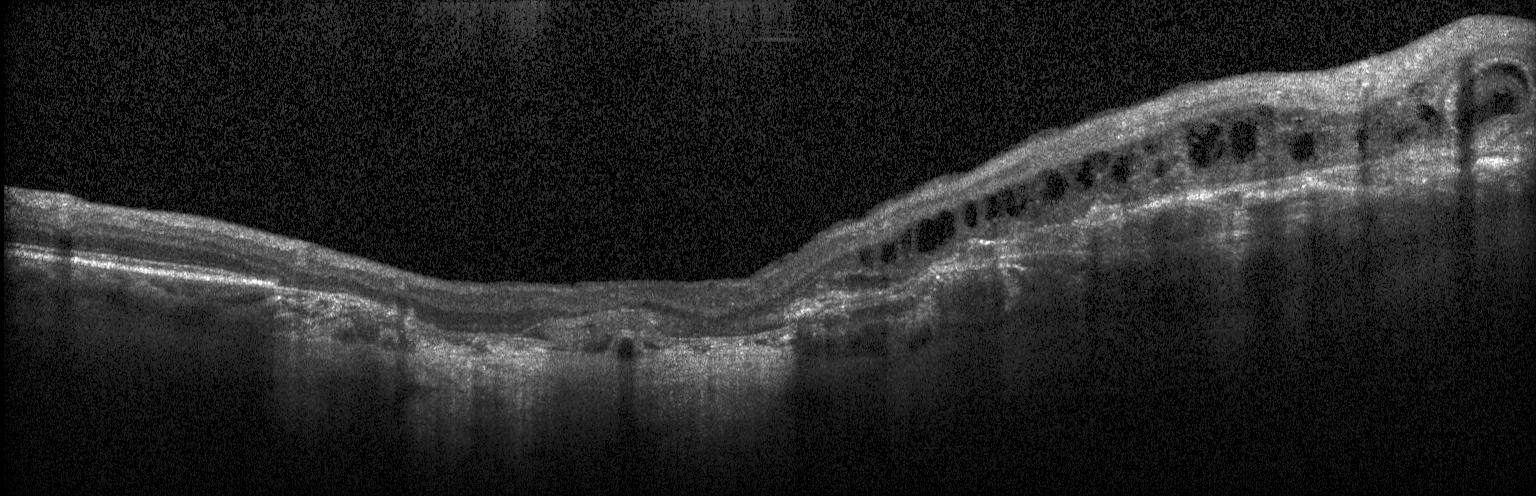

Retinal OCT B-scan. Instrument: Heidelberg Spectralis. SD-OCT
This B-scan demonstrates a choroidal neovascular membrane.